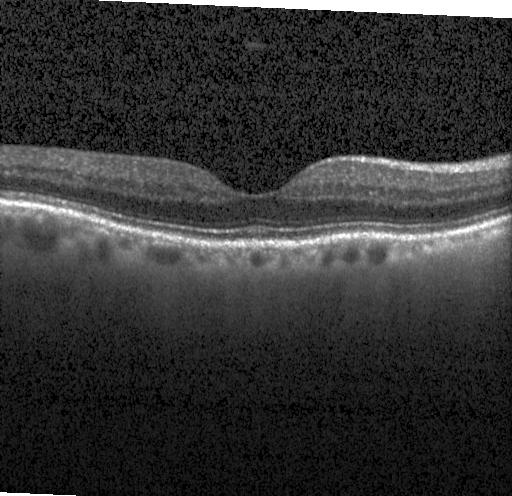
Retinal OCT B-scan, Heidelberg Spectralis, fovea-centered, spectral-domain optical coherence tomography. Dx: neither choroidal neovascularization, diabetic macular edema, nor drusen.